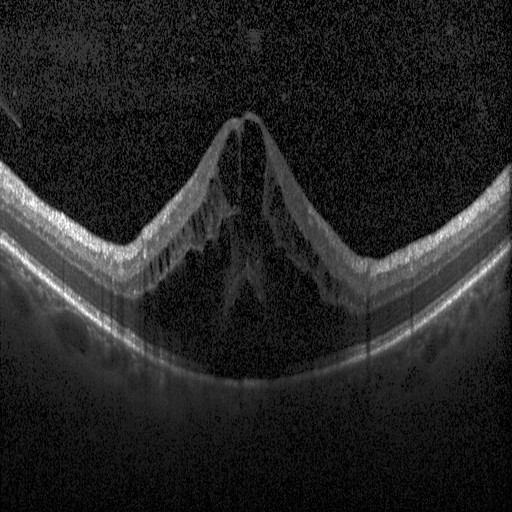

Retinal OCT cross-section, horizontal scan through the fovea, Heidelberg Spectralis.
Dx: diabetic macular edema (DME).